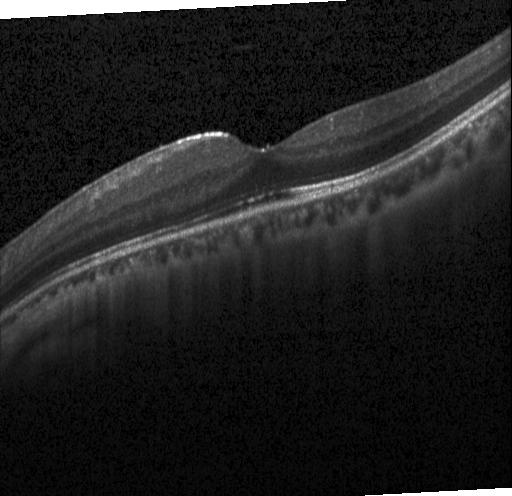 Retinal OCT B-scan. Centered on the fovea. Acquired on a Heidelberg Spectralis
Finding: no evidence of choroidal neovascularization, diabetic macular edema, or drusen.